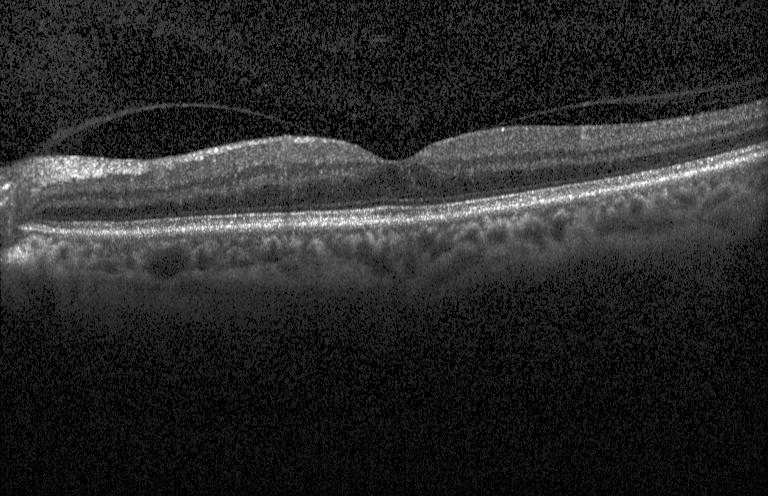

This B-scan demonstrates no CNV, DME, or drusen.